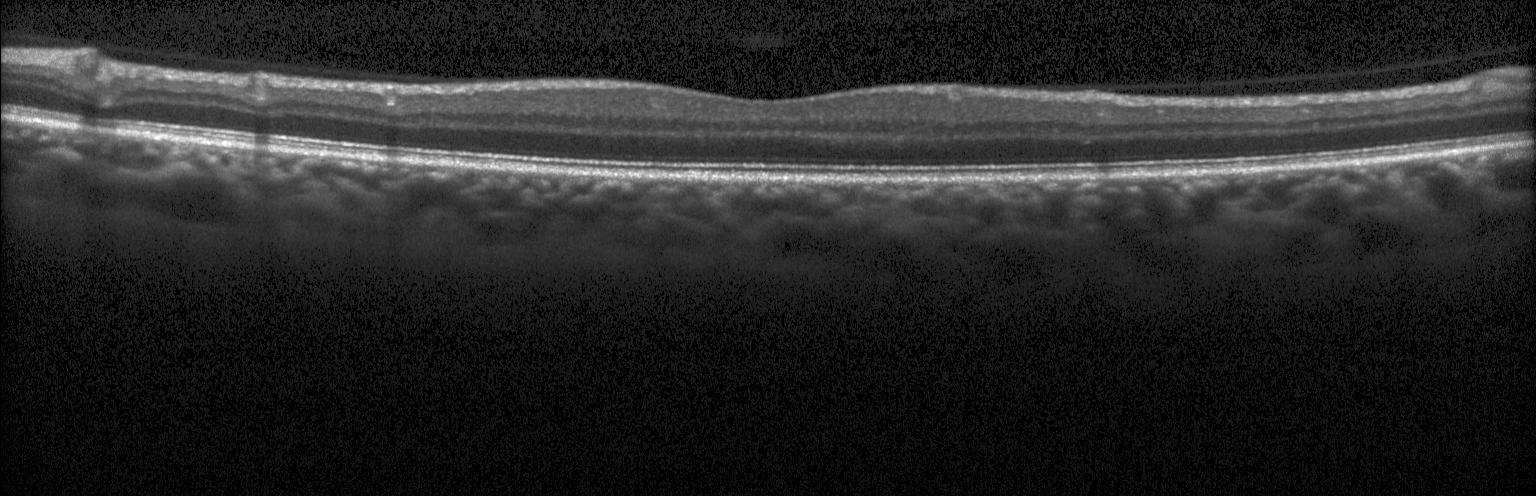 Finding: no evidence of choroidal neovascularization, diabetic macular edema, or drusen.